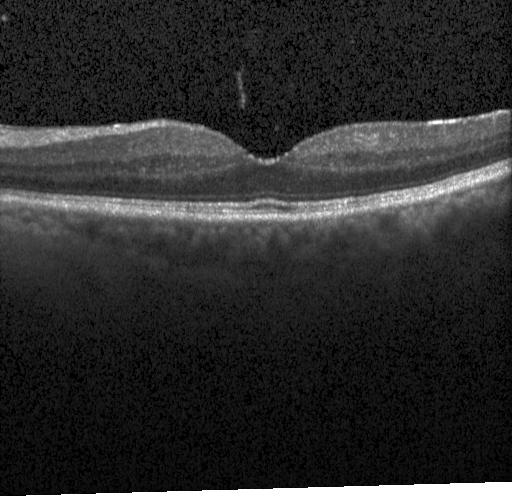
Impression: neither CNV, DME, nor drusen.